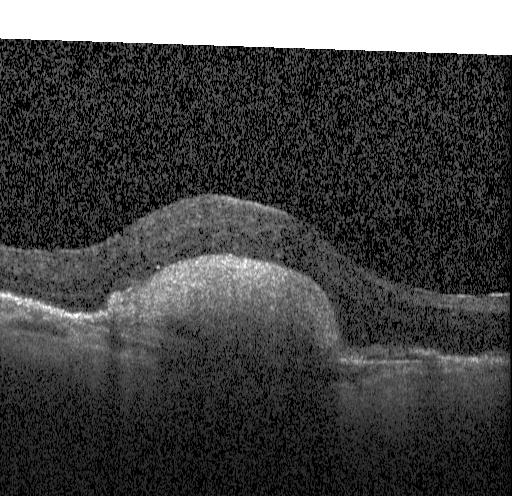 Fovea-centered, optical coherence tomography B-scan, spectral-domain OCT, Heidelberg Spectralis. Diagnosis: CNV.